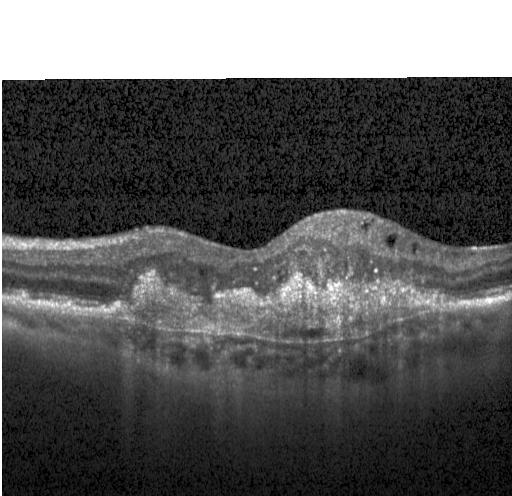 Optical coherence tomography B-scan, macular scan — Impression: a choroidal neovascular membrane.